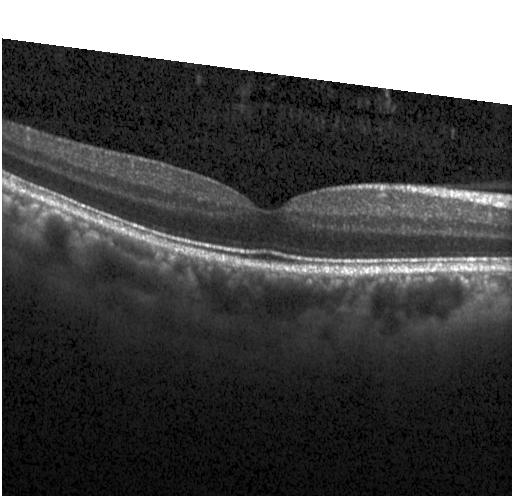 Optical coherence tomography B-scan.
Impression: no evidence of choroidal neovascularization, diabetic macular edema, or drusen.